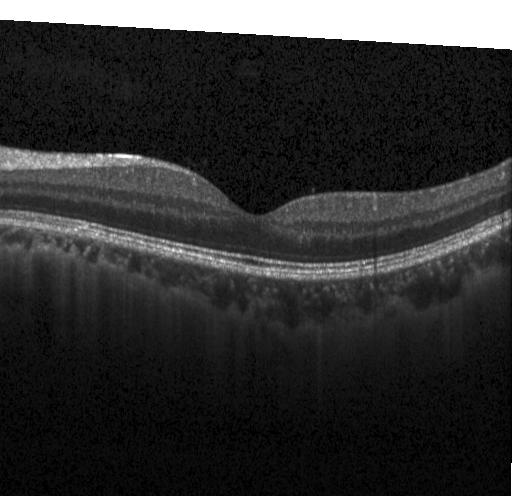
Impression: no choroidal neovascularization, no diabetic macular edema, and no drusen.